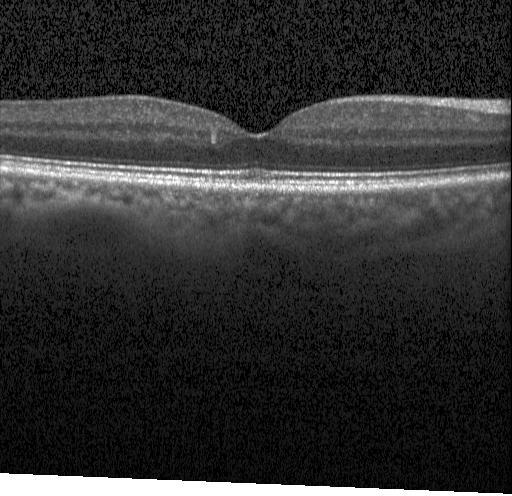
OCT finding: no evidence of choroidal neovascularization, diabetic macular edema, or drusen.